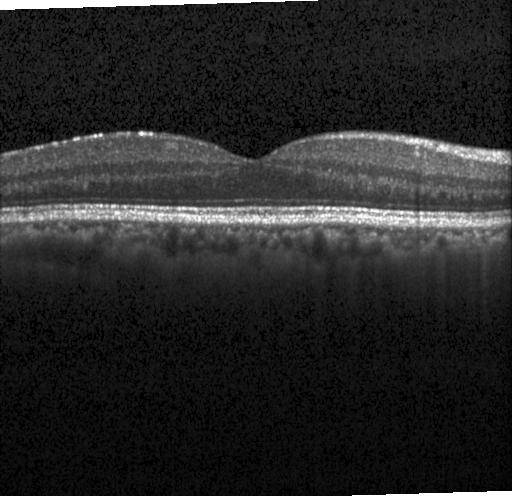 Optical coherence tomography B-scan, Heidelberg Spectralis, spectral-domain OCT, fovea-centered — Macular OCT: no choroidal neovascularization, diabetic macular edema, or drusen.